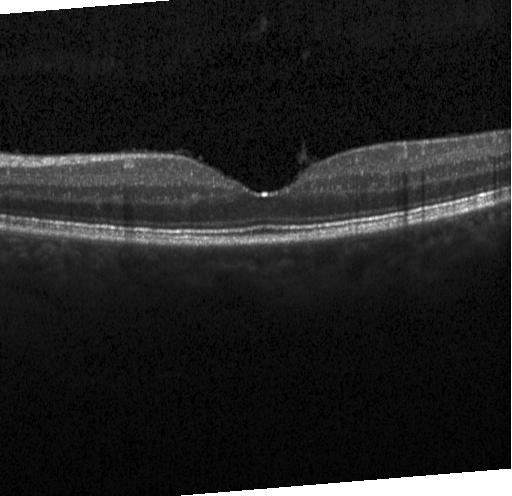
Spectral-domain optical coherence tomography, OCT line scan
This B-scan demonstrates neither choroidal neovascularization, diabetic macular edema, nor drusen.